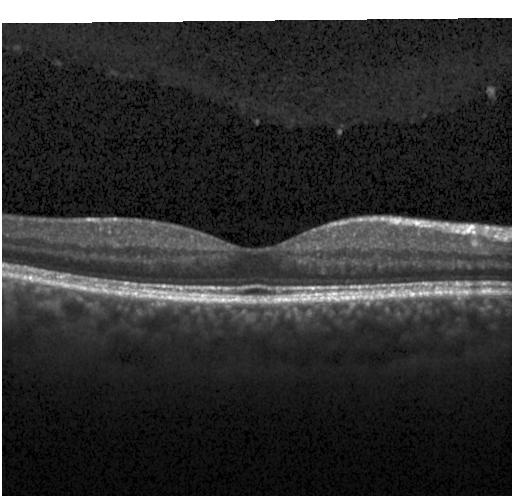
OCT line scan — Macular OCT: no evidence of choroidal neovascularization, diabetic macular edema, or drusen.